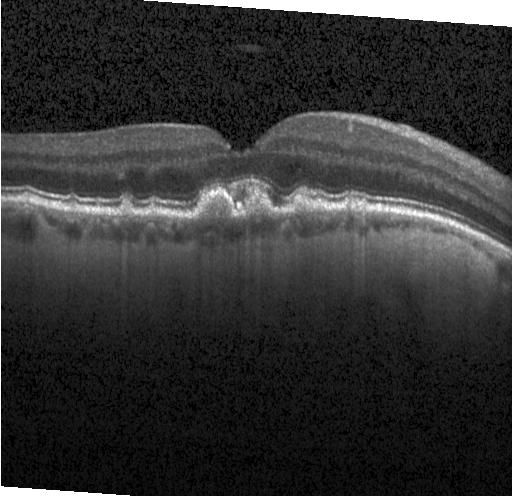

Retinal OCT B-scan.
Assessment: multiple drusen.